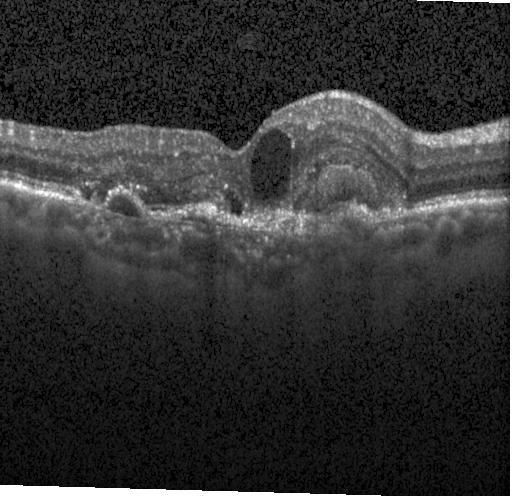

Spectral-domain OCT; OCT B-scan; macular scan. The scan shows a choroidal neovascular membrane.